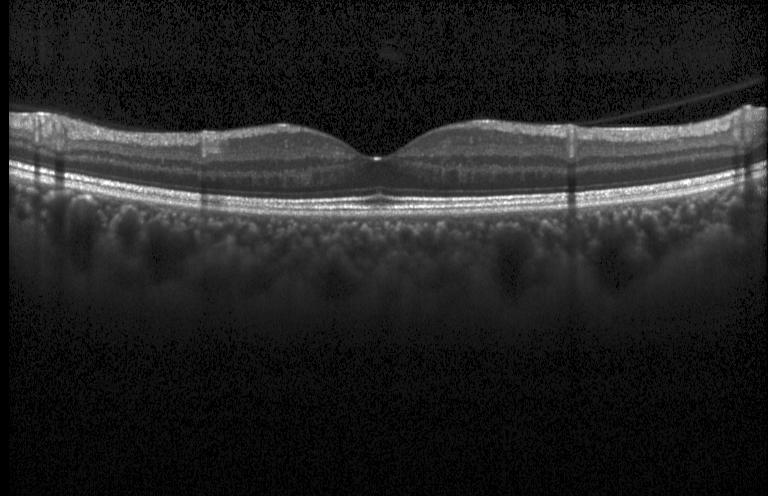
Optical coherence tomography scan, through the macula. Finding: neither choroidal neovascularization, diabetic macular edema, nor drusen.